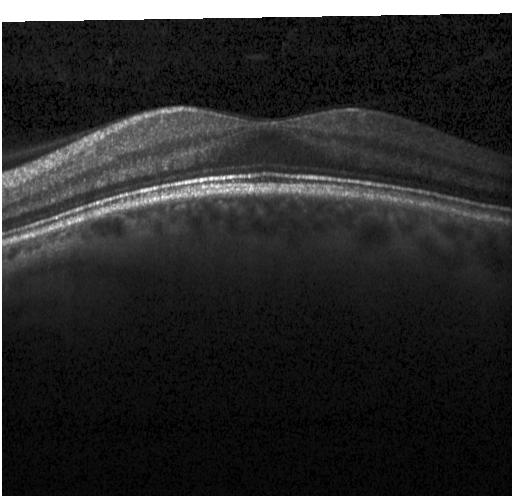
Finding: neither choroidal neovascularization, diabetic macular edema, nor drusen.